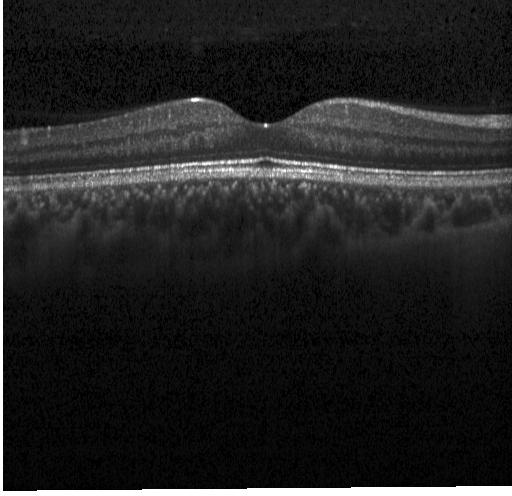

Spectral-domain OCT. Optical coherence tomography B-scan — Diagnosis: no evidence of choroidal neovascularization, diabetic macular edema, or drusen.